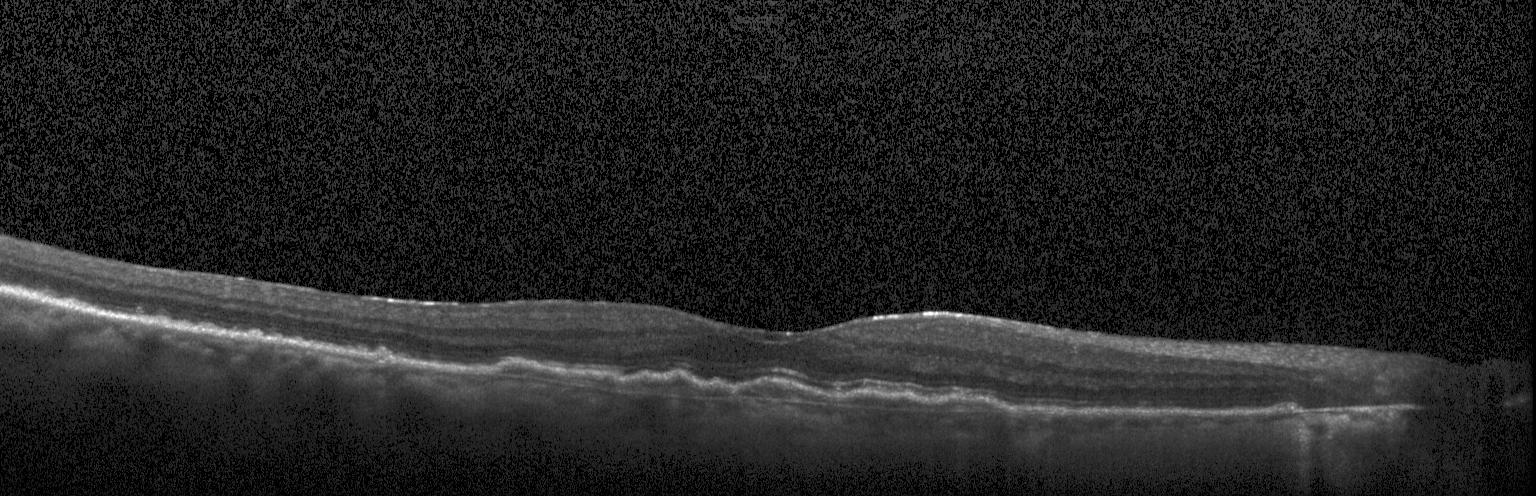 OCT line scan, spectral-domain OCT, through the macula, Heidelberg Spectralis OCT system. This B-scan demonstrates a choroidal neovascular membrane.